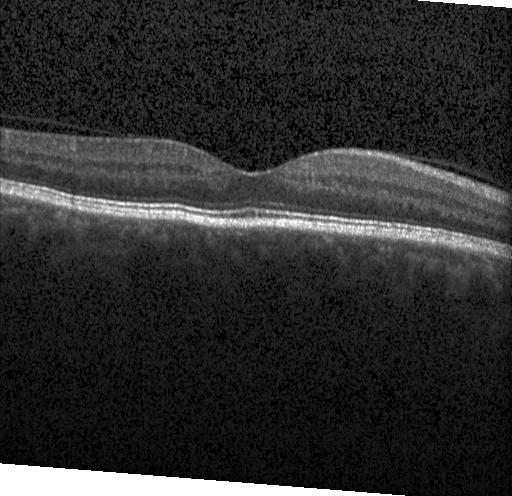

OCT B-scan. Spectral-domain OCT. Instrument: Heidelberg Spectralis. Horizontal scan through the fovea. Impression: no choroidal neovascularization, diabetic macular edema, or drusen.